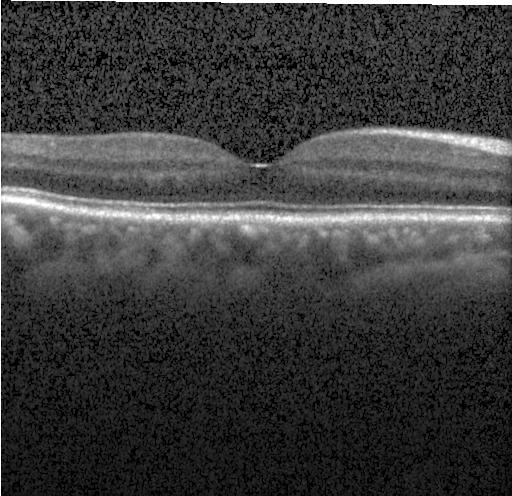

Dx: no CNV, DME, or drusen.